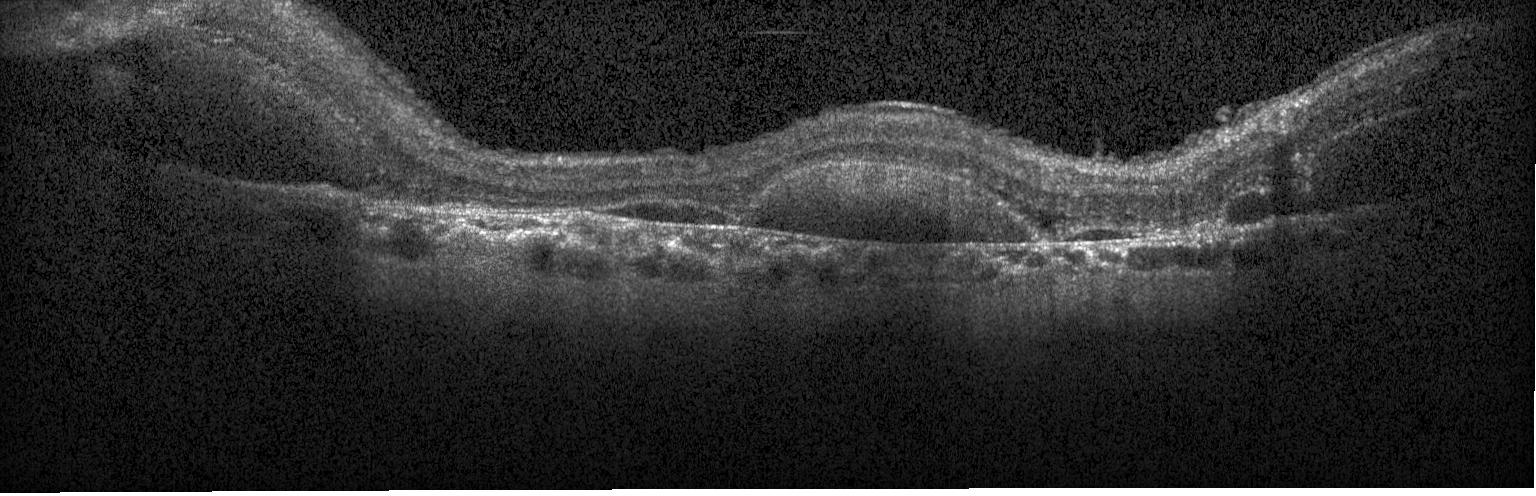

OCT line scan
Impression: CNV.